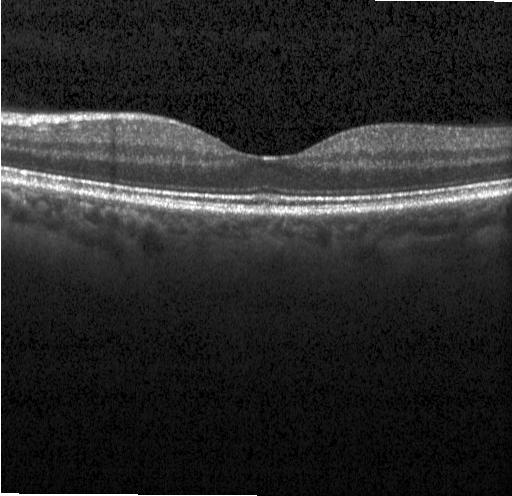
Optical coherence tomography scan; macular scan. Assessment: no evidence of choroidal neovascularization, diabetic macular edema, or drusen.